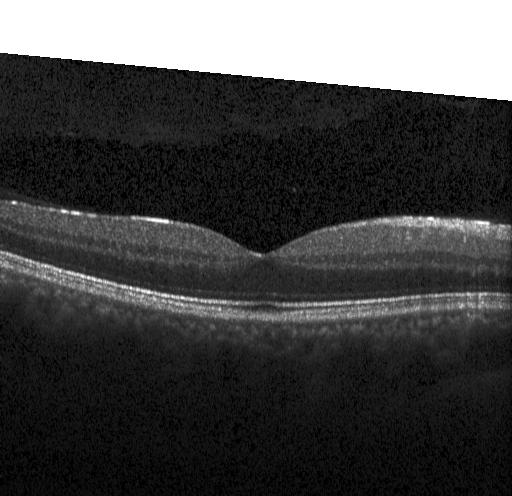

Retinal OCT cross-section showing neither CNV, DME, nor drusen.